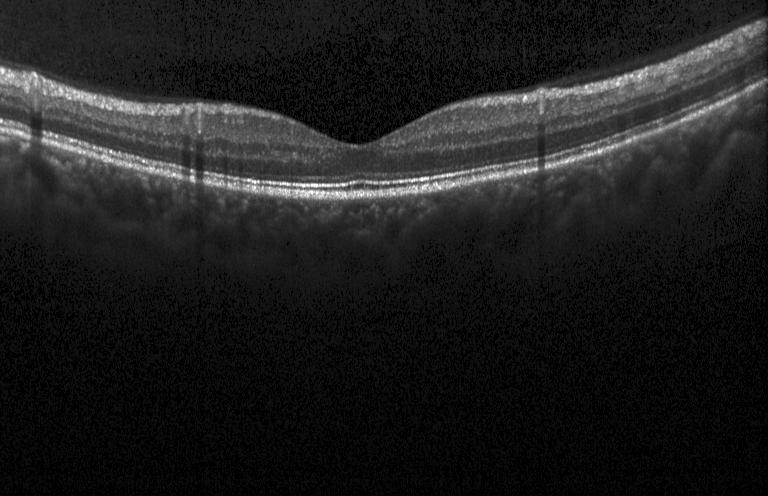
Retinal OCT B-scan · fovea-centered
Macular OCT: no CNV, no DME, and no drusen.